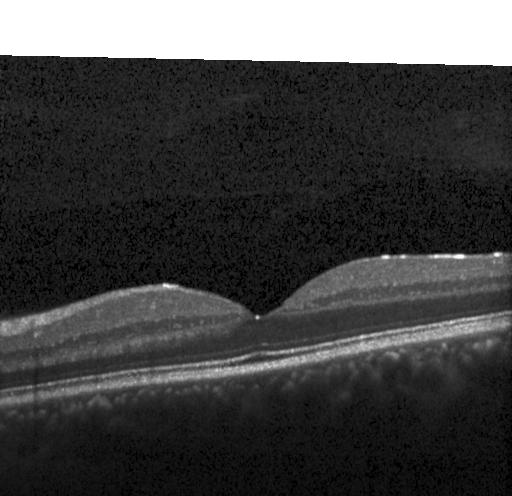 Diagnosis: no CNV, no DME, and no drusen.